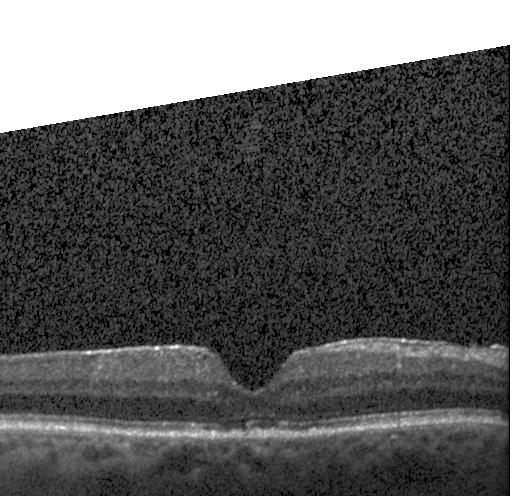

Acquired on a Heidelberg Spectralis · fovea-centered · spectral-domain OCT · retinal OCT cross-section. Finding: no evidence of choroidal neovascularization, diabetic macular edema, or drusen.